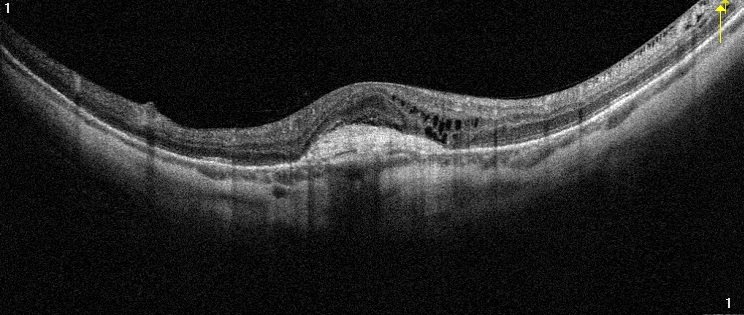

Retinal OCT cross-section. Optovue Avanti RTVue XR. Fovea-centered
Assessment: AMD.